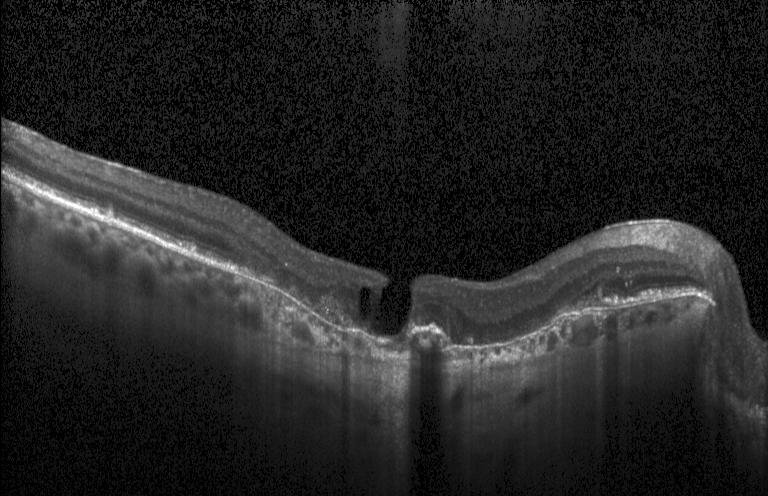 Fovea-centered · OCT B-scan — Impression: choroidal neovascularization (CNV).